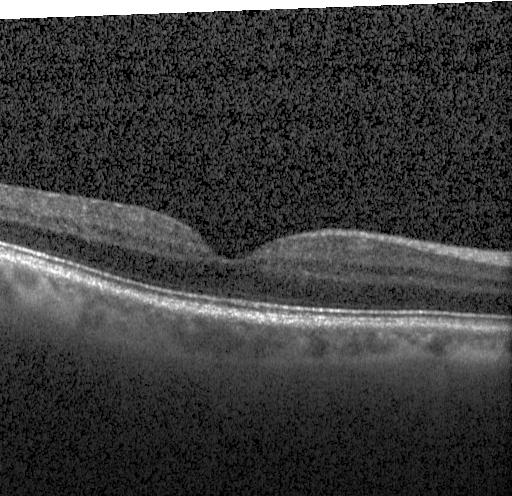 Dx: no evidence of CNV, DME, or drusen.